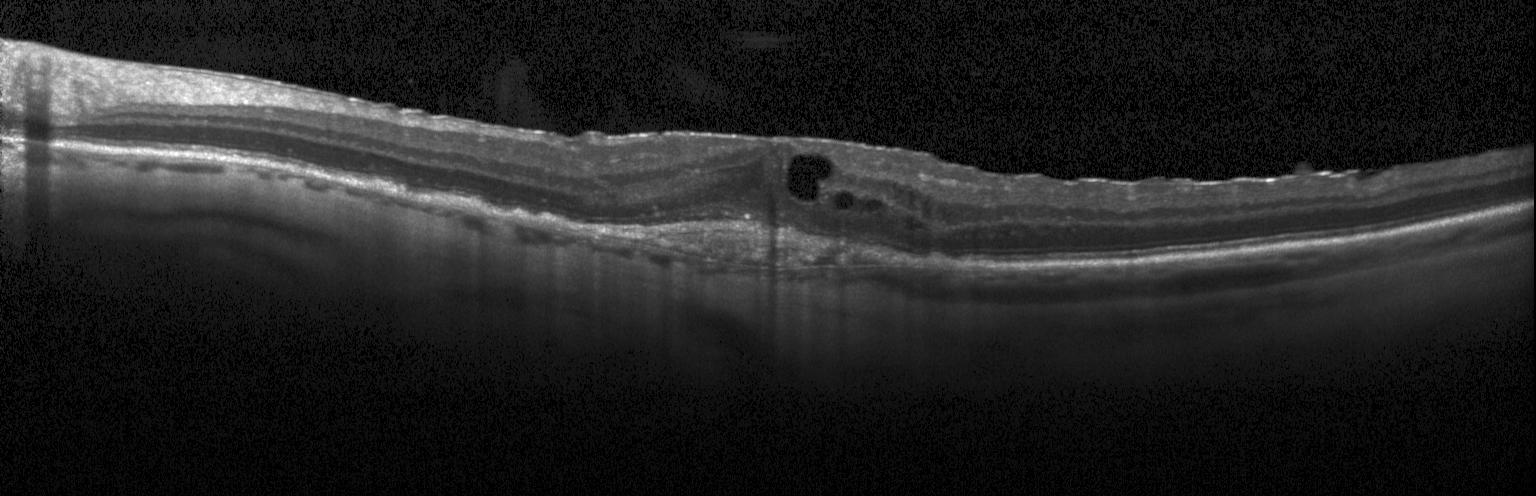 Dx: a choroidal neovascular membrane.